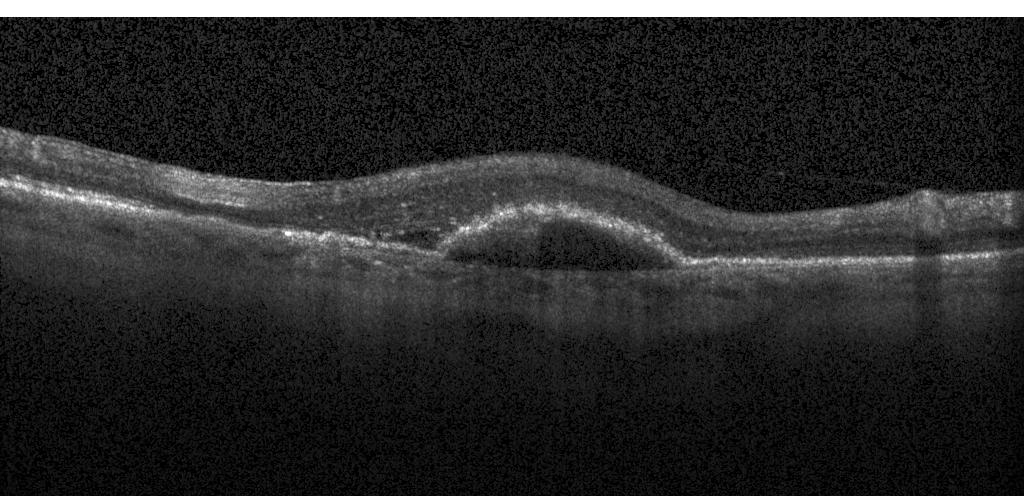
Instrument: Heidelberg Spectralis; optical coherence tomography scan — Diagnosis: choroidal neovascularization.